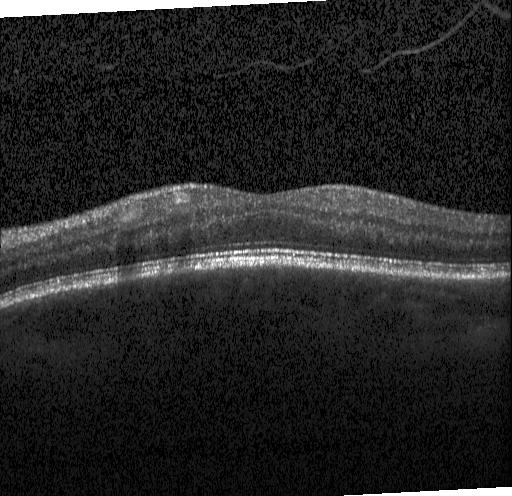

Centered on the fovea. Instrument: Heidelberg Spectralis. Retinal OCT cross-section. Diagnosis: no evidence of choroidal neovascularization, diabetic macular edema, or drusen.